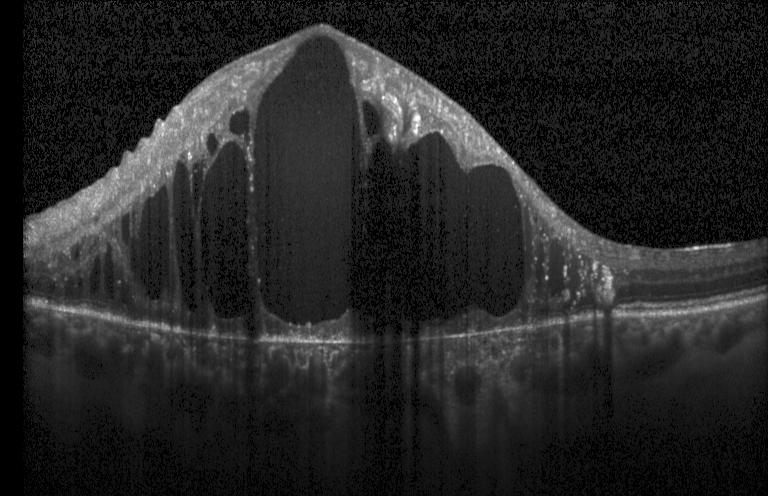

Macular OCT: diabetic macular edema.